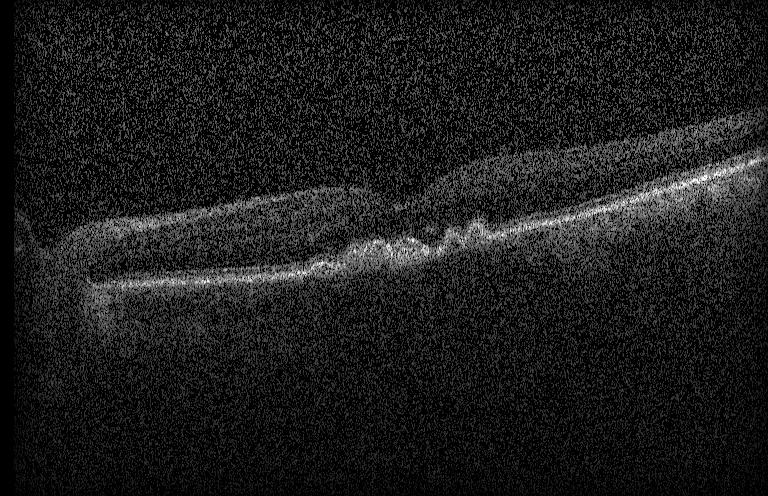 Fovea-centered, instrument: Heidelberg Spectralis, spectral-domain OCT, optical coherence tomography B-scan
Finding: choroidal neovascularization (CNV).